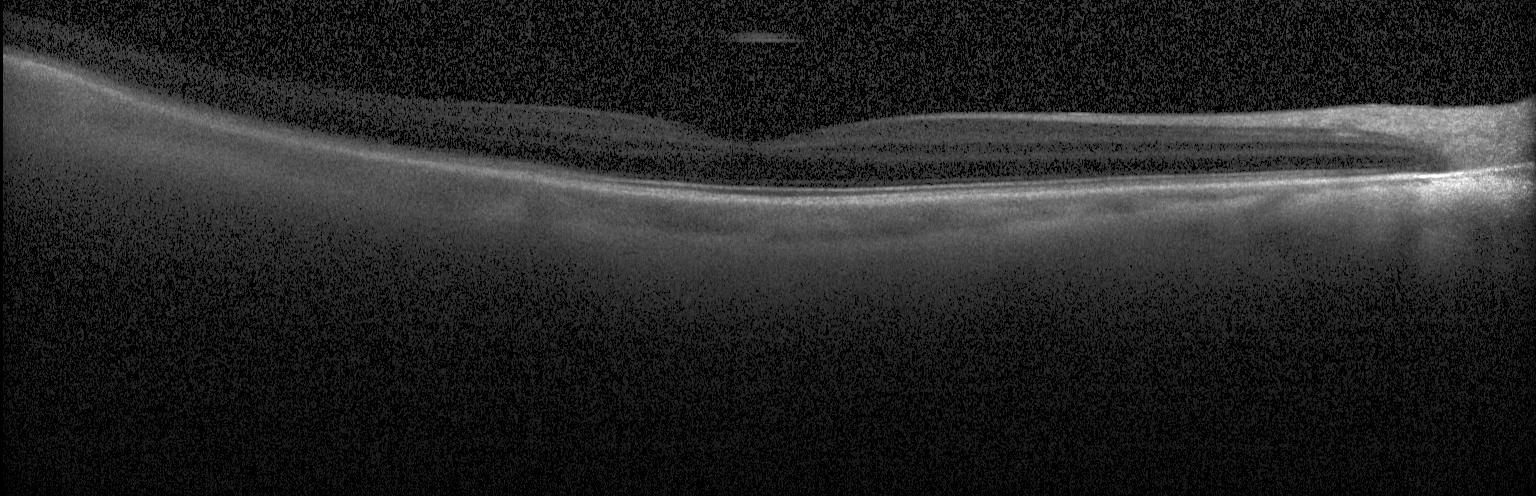 Dx: no CNV, no DME, and no drusen.